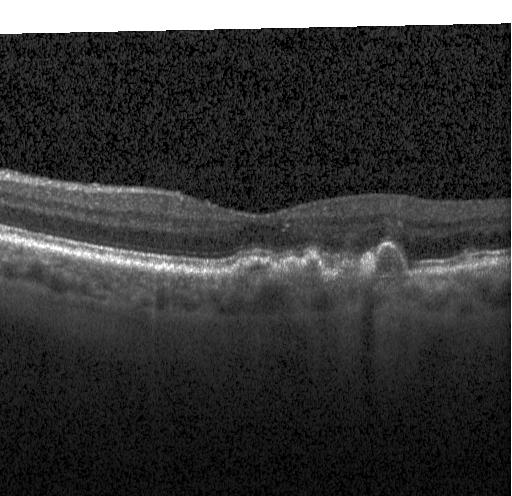

OCT B-scan, Heidelberg Spectralis OCT system, spectral-domain OCT.
Diagnosis: multiple drusen.